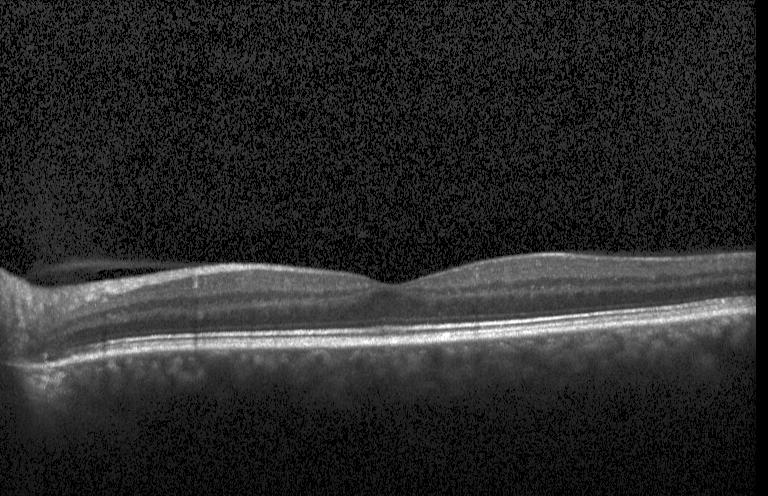
Finding: no evidence of choroidal neovascularization, diabetic macular edema, or drusen.